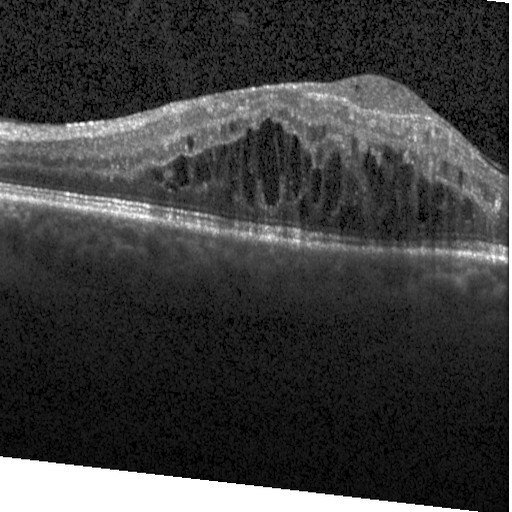

OCT B-scan — The scan shows diabetic macular edema.